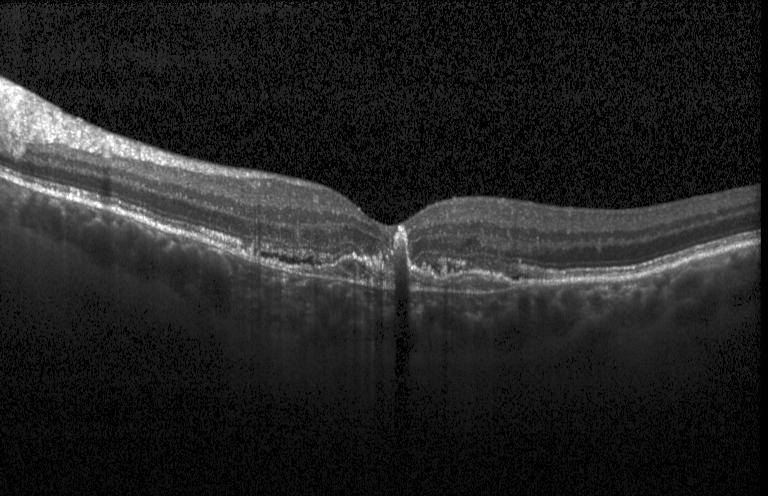

Finding: a choroidal neovascular membrane.